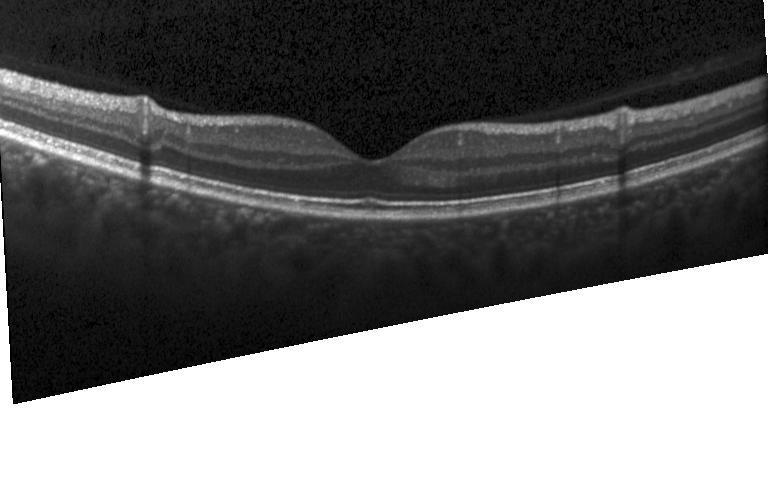
Dx: no choroidal neovascularization, no diabetic macular edema, and no drusen.